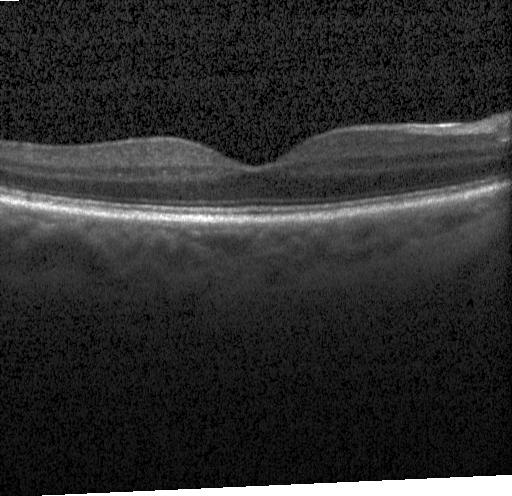
Optical coherence tomography B-scan; Heidelberg Spectralis OCT system — Assessment: neither choroidal neovascularization, diabetic macular edema, nor drusen.